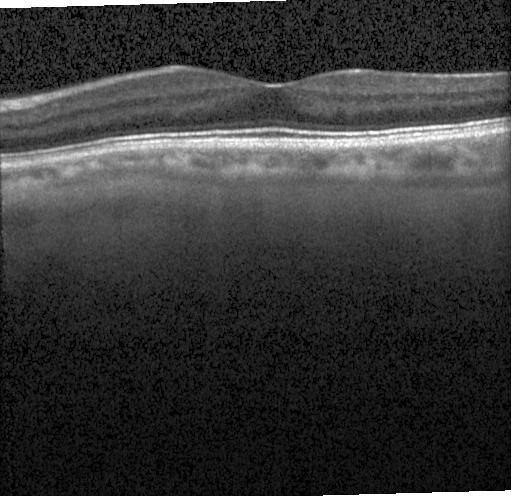 Retinal OCT cross-section.
This B-scan demonstrates no evidence of choroidal neovascularization, diabetic macular edema, or drusen.